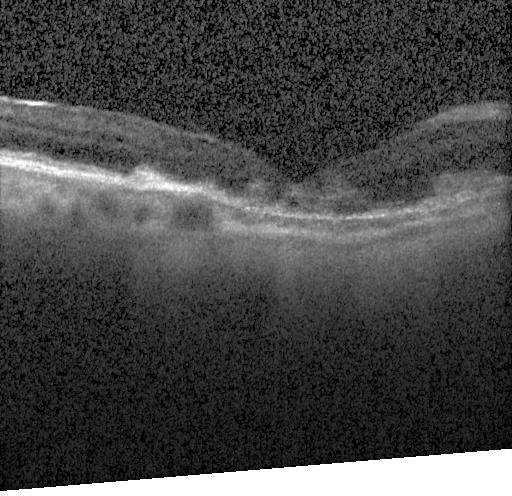
Through the macula · instrument: Heidelberg Spectralis · SD-OCT · OCT B-scan. Diagnosis: choroidal neovascularization.